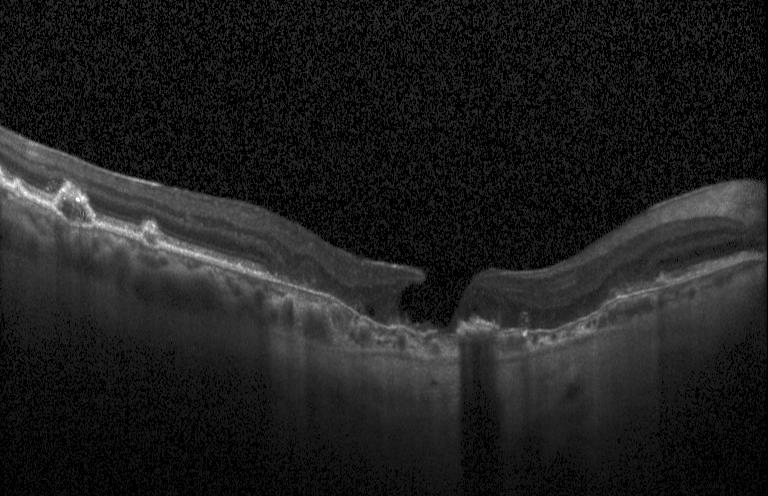 Retinal OCT cross-section
This B-scan demonstrates a choroidal neovascular membrane.